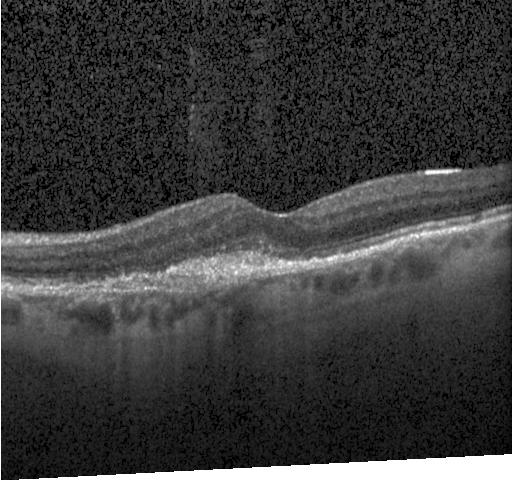
Optical coherence tomography scan; Heidelberg Spectralis; horizontal scan through the fovea; spectral-domain OCT. Dx: choroidal neovascularization (CNV).